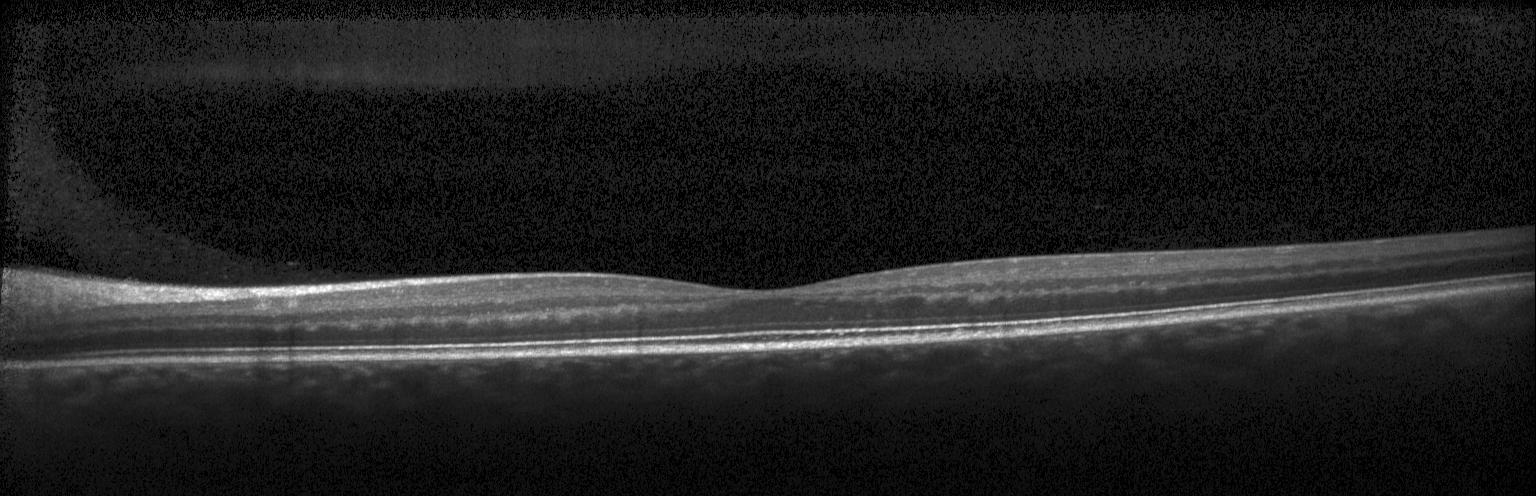

Retinal OCT cross-section.
Assessment: no evidence of choroidal neovascularization, diabetic macular edema, or drusen.